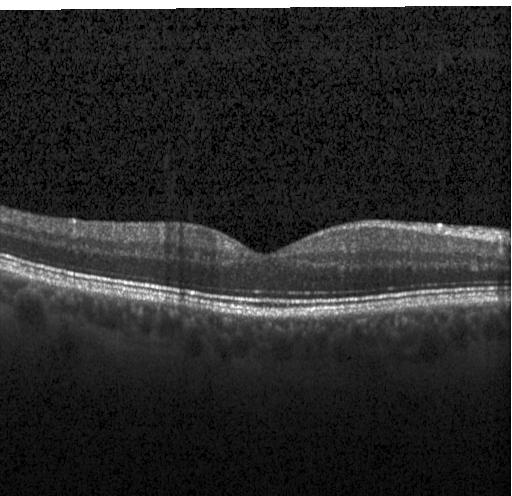
Diagnosis: no CNV, DME, or drusen.